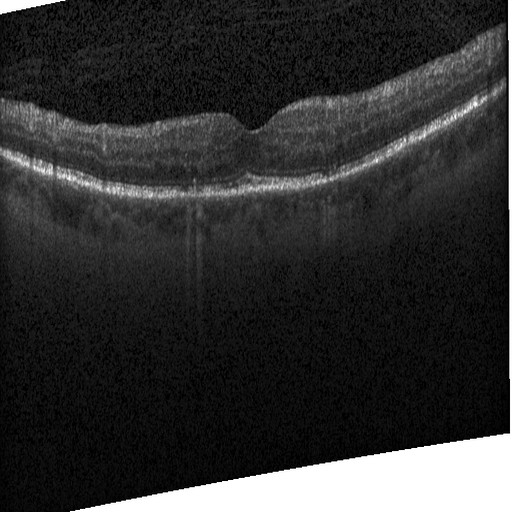

Finding: diabetic macular edema.